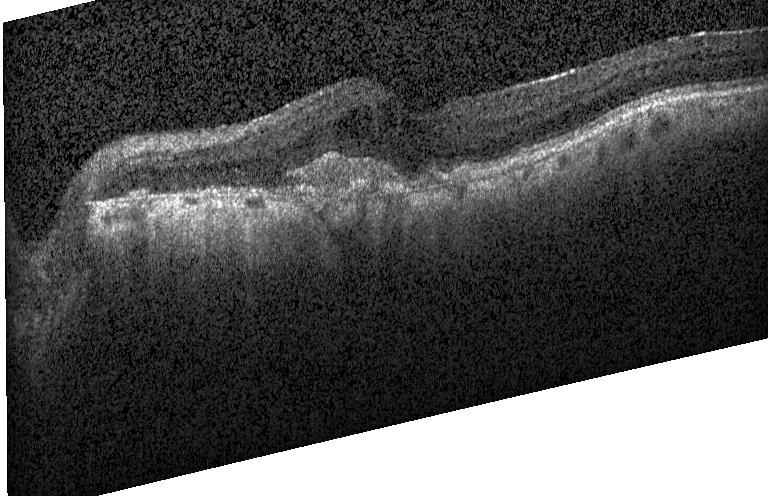

Optical coherence tomography B-scan
OCT finding: choroidal neovascularization (CNV).